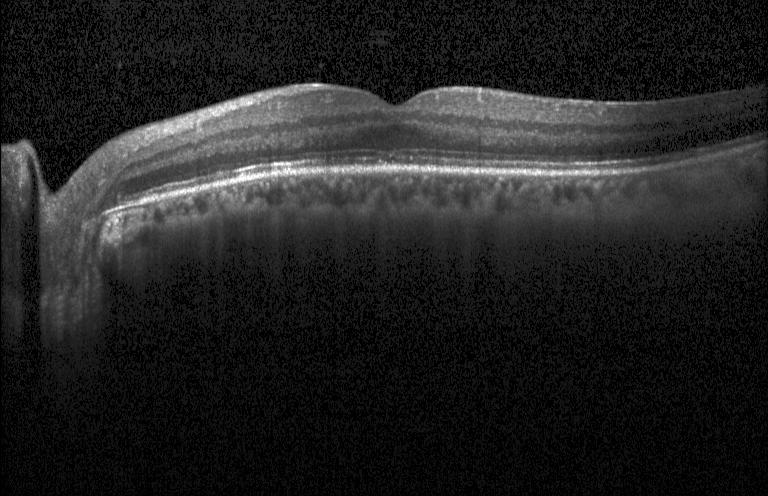
Finding: neither choroidal neovascularization, diabetic macular edema, nor drusen.